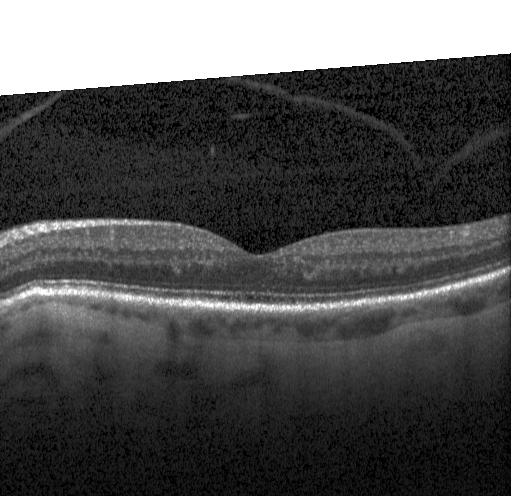

Heidelberg Spectralis · OCT B-scan · horizontal scan through the fovea.
Impression: no evidence of CNV, DME, or drusen.